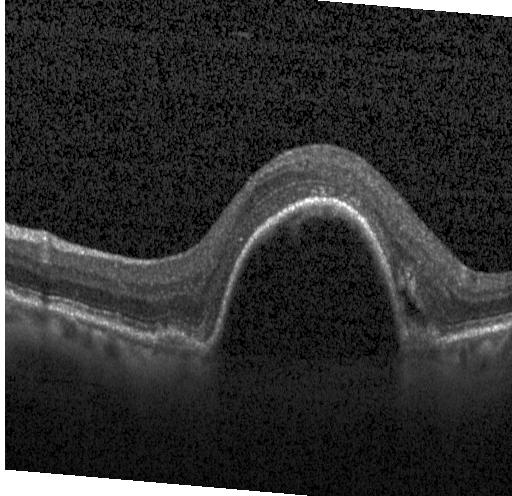 Spectral-domain OCT; horizontal scan through the fovea; Heidelberg Spectralis OCT system; retinal OCT B-scan
Impression: choroidal neovascularization.